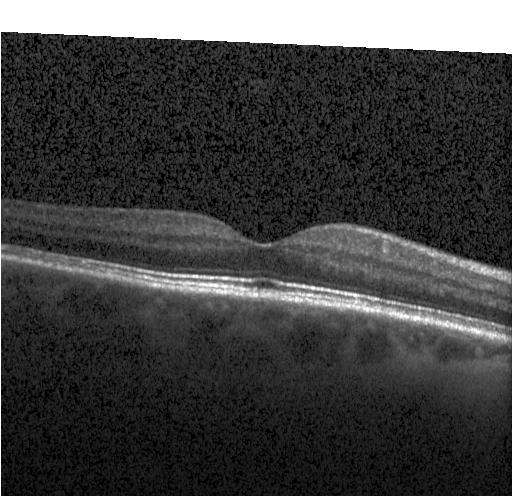

Heidelberg Spectralis, through the macula, retinal OCT B-scan. This B-scan demonstrates no choroidal neovascularization, diabetic macular edema, or drusen.